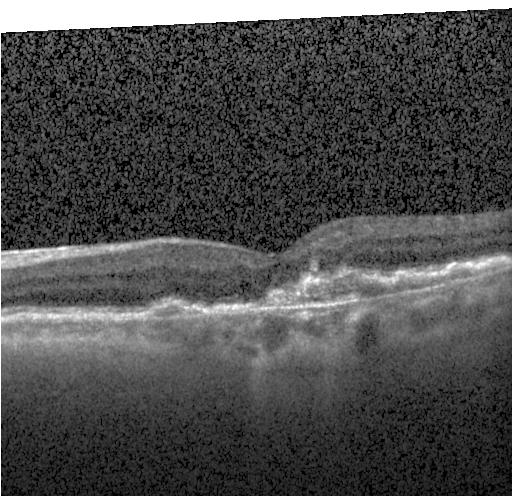 Diagnosis: choroidal neovascularization.